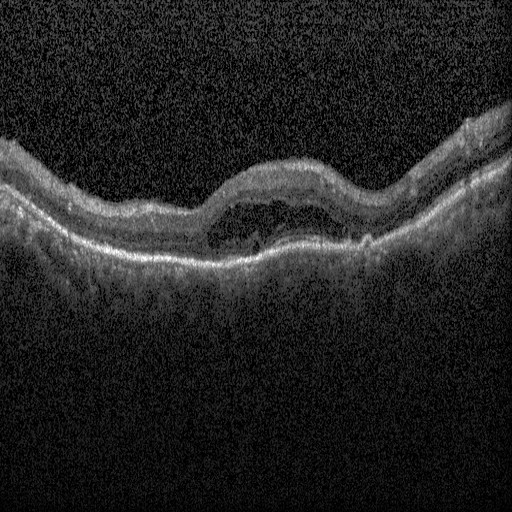 SD-OCT, OCT line scan — Diabetic macular edema.